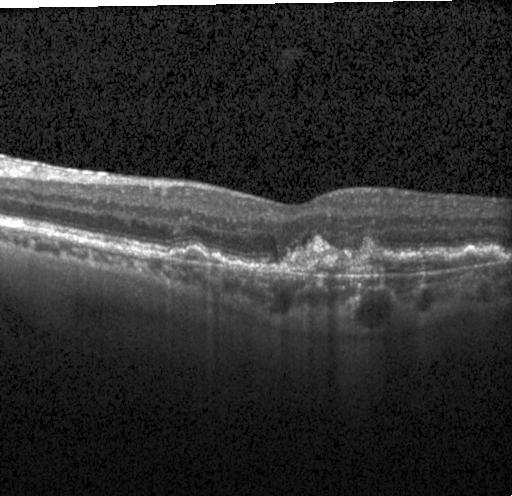 Retinal OCT cross-section · macular scan · SD-OCT.
Finding: choroidal neovascularization (CNV).